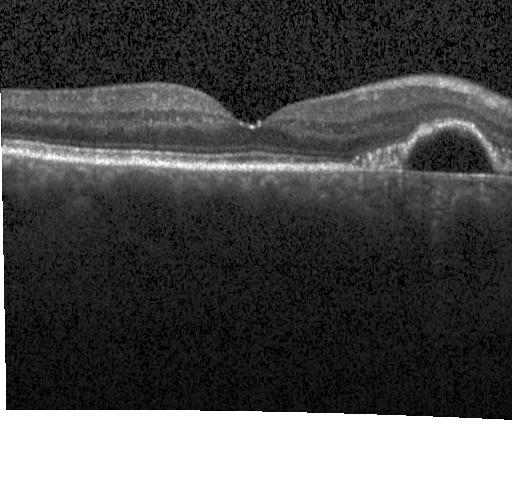
Finding: choroidal neovascularization (CNV).